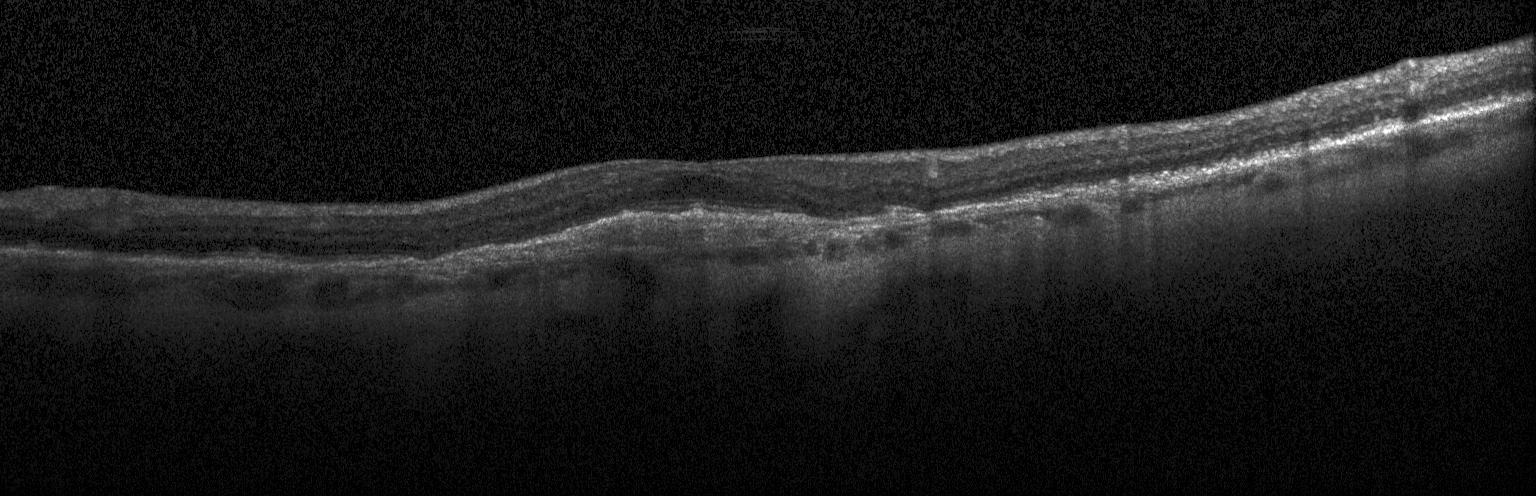

OCT line scan · fovea-centered · acquired on a Heidelberg Spectralis · SD-OCT — Finding: choroidal neovascularization.